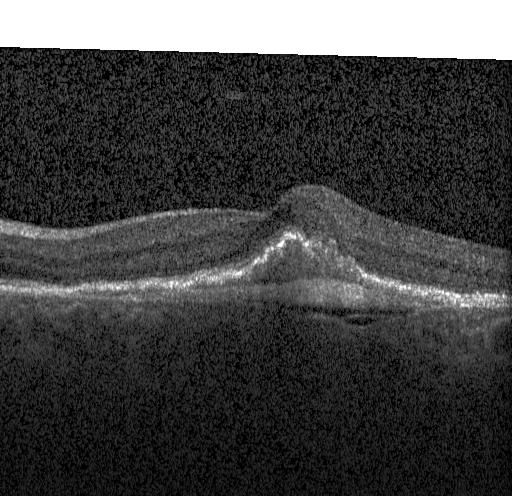

Heidelberg Spectralis OCT system · spectral-domain OCT · retinal OCT cross-section · horizontal scan through the fovea. OCT finding: a choroidal neovascular membrane.